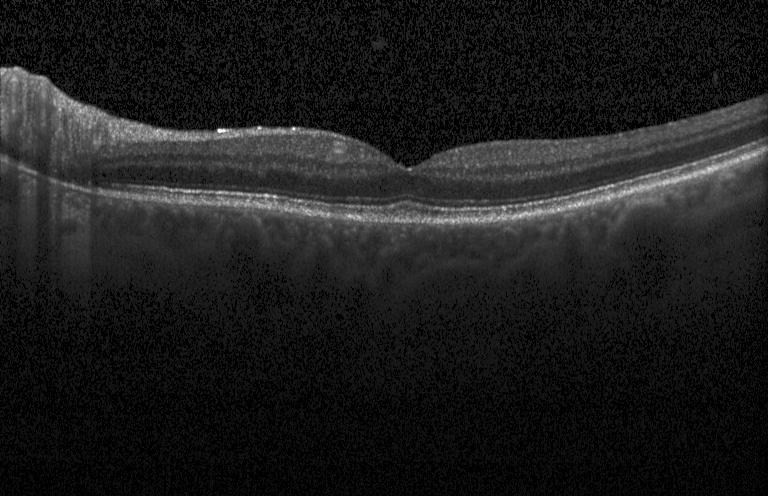
Retinal OCT B-scan, Heidelberg Spectralis. Diagnosis: no choroidal neovascularization, no diabetic macular edema, and no drusen.